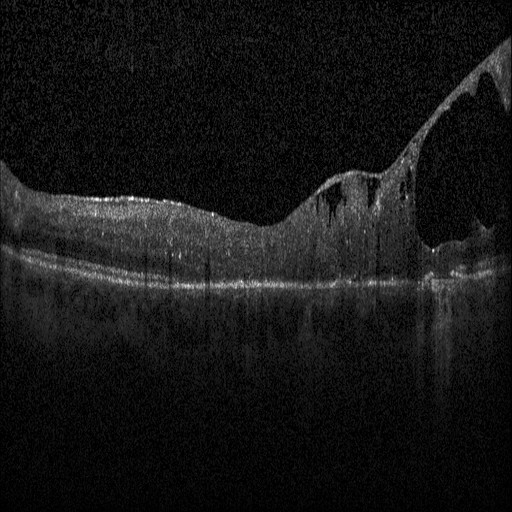
Retinal OCT B-scan. Impression: diabetic macular edema (DME).